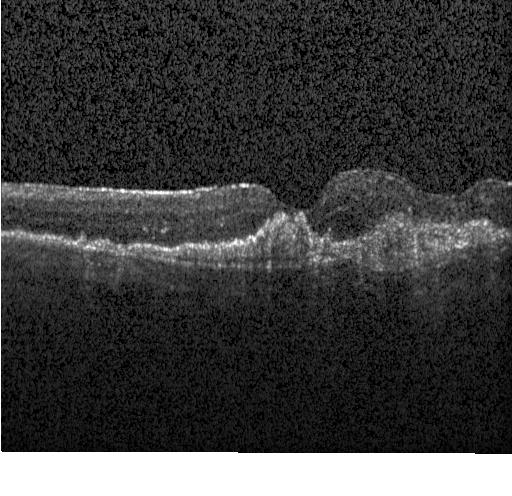 Spectral-domain OCT. Heidelberg Spectralis. Retinal OCT B-scan. Centered on the fovea — The scan shows choroidal neovascularization.